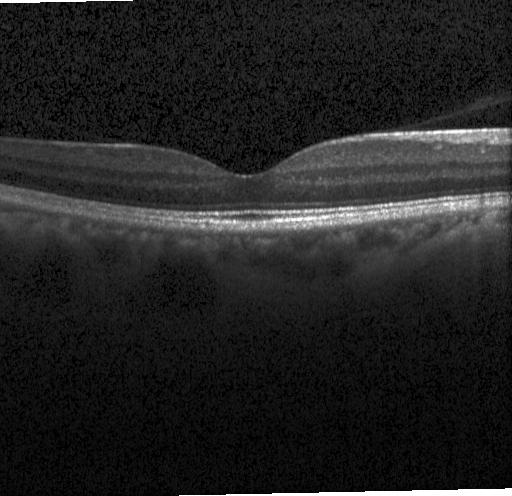

Impression: no choroidal neovascularization, no diabetic macular edema, and no drusen.